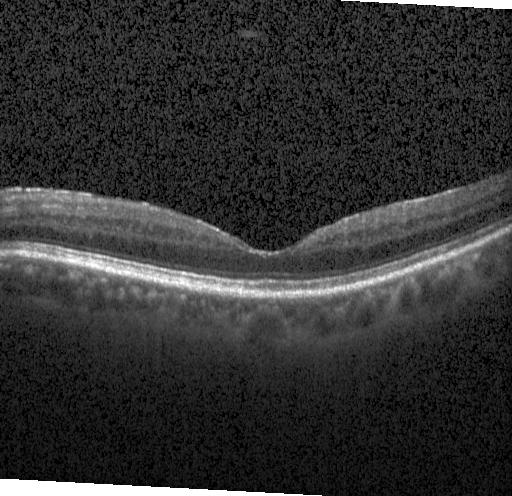

Through the macula, OCT line scan, spectral-domain optical coherence tomography, Heidelberg Spectralis OCT system — This B-scan demonstrates neither choroidal neovascularization, diabetic macular edema, nor drusen.